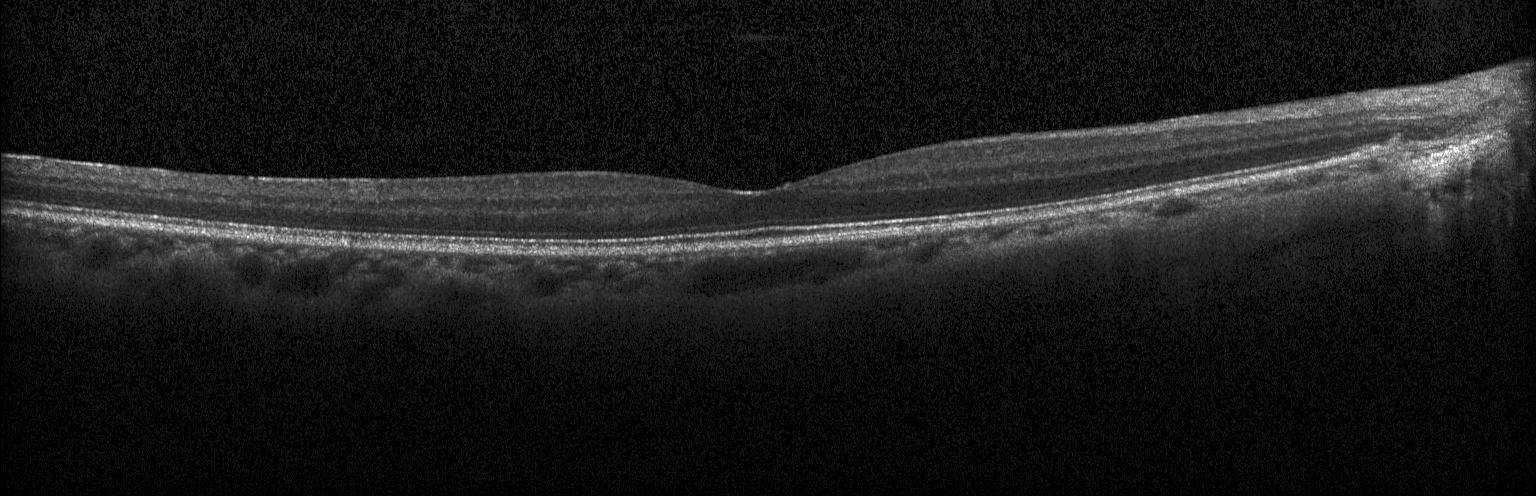 OCT B-scan · spectral-domain optical coherence tomography · horizontal scan through the fovea — Macular OCT: neither CNV, DME, nor drusen.